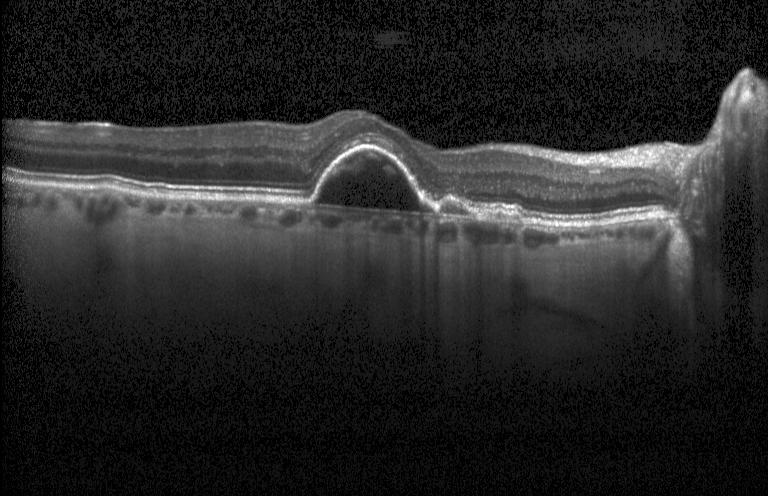 Centered on the fovea; OCT B-scan — Diagnosis: a choroidal neovascular membrane.